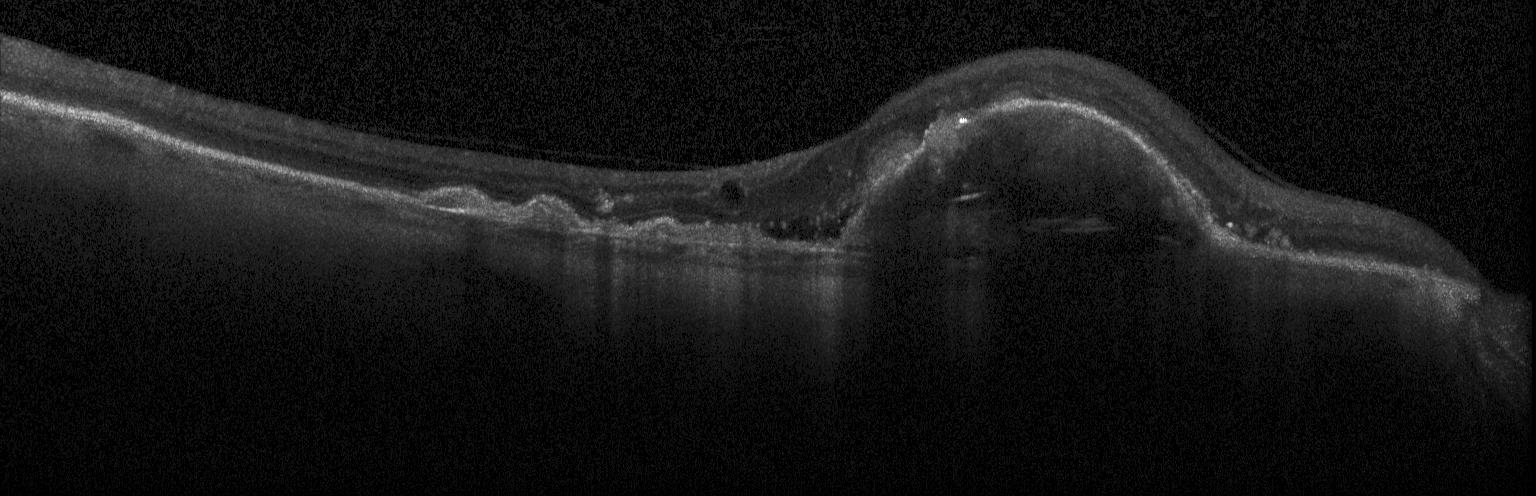

Retinal OCT cross-section. Centered on the fovea. Acquired on a Heidelberg Spectralis. Spectral-domain OCT.
Finding: a choroidal neovascular membrane.